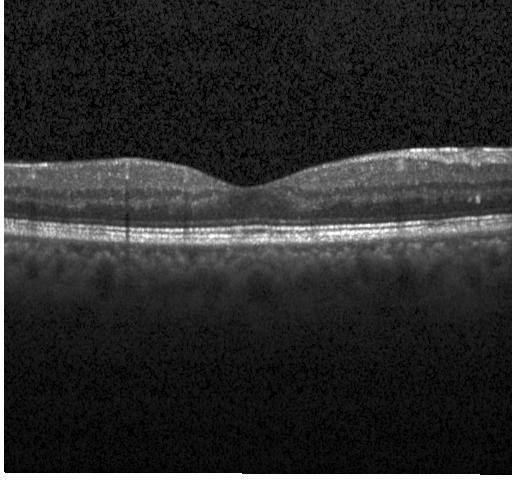
Macular OCT demonstrating no evidence of choroidal neovascularization, diabetic macular edema, or drusen.